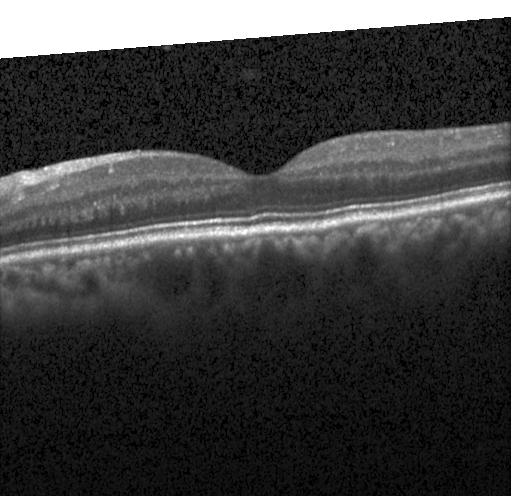

OCT B-scan; Heidelberg Spectralis OCT system; SD-OCT — Macular OCT: no evidence of CNV, DME, or drusen.